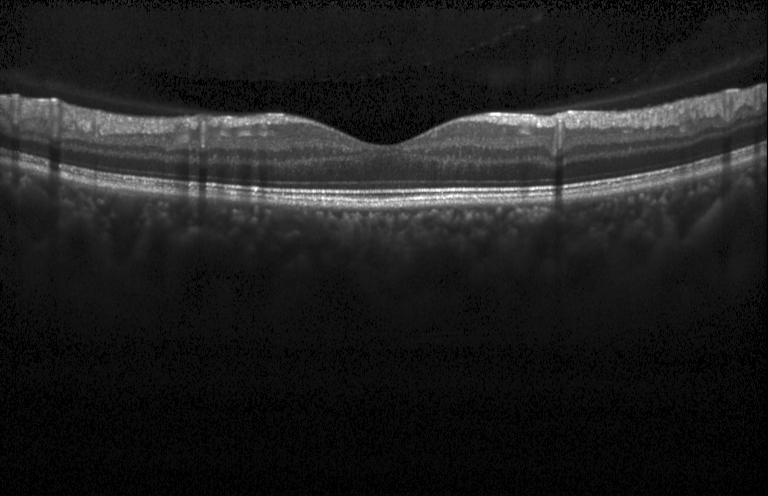 OCT B-scan
Macular OCT: no choroidal neovascularization, no diabetic macular edema, and no drusen.